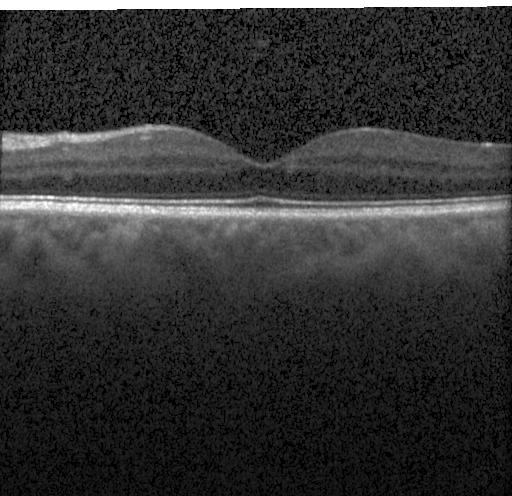 Finding: no evidence of choroidal neovascularization, diabetic macular edema, or drusen.